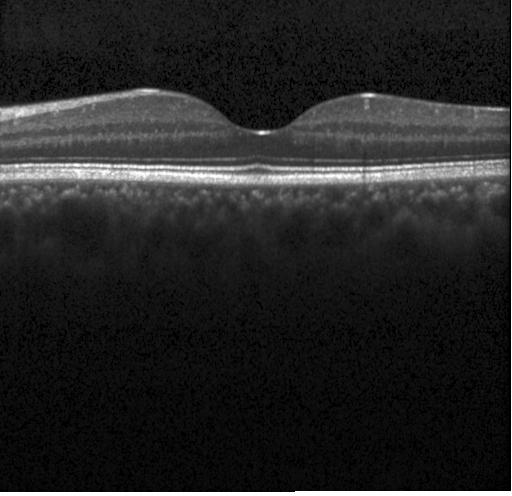 Retinal OCT cross-section; fovea-centered; SD-OCT; Heidelberg Spectralis.
Finding: no evidence of CNV, DME, or drusen.